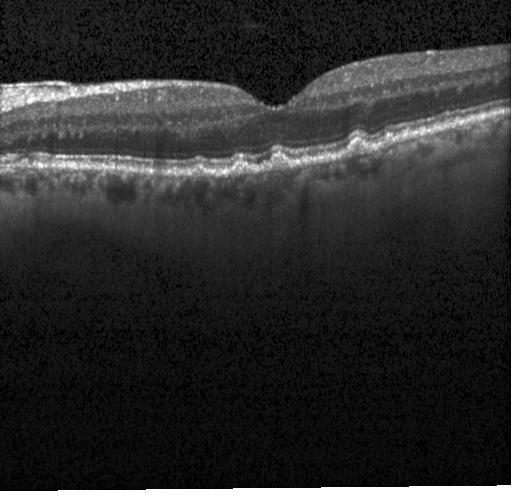

Through the macula; retinal OCT cross-section
Impression: multiple drusen.